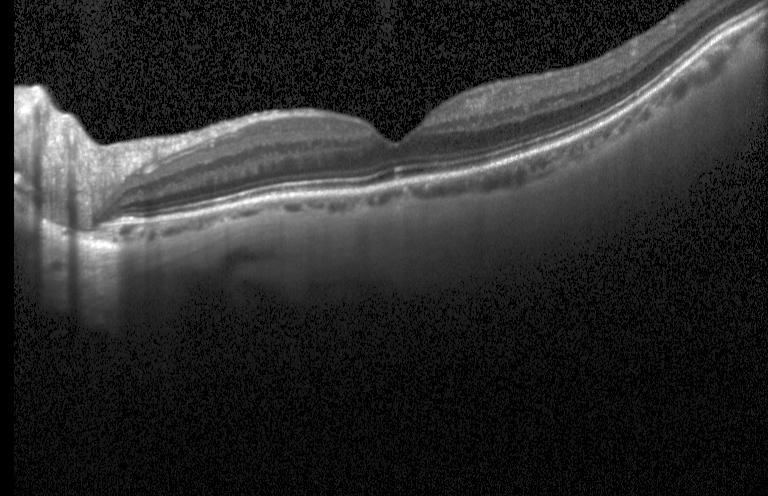
OCT finding: no CNV, DME, or drusen.